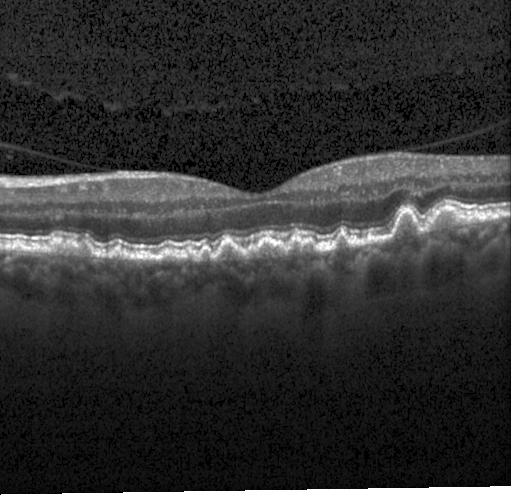

OCT scan showing drusen.